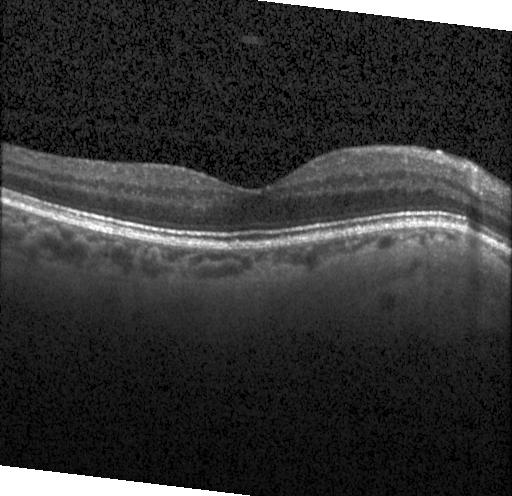

The scan shows no evidence of choroidal neovascularization, diabetic macular edema, or drusen.